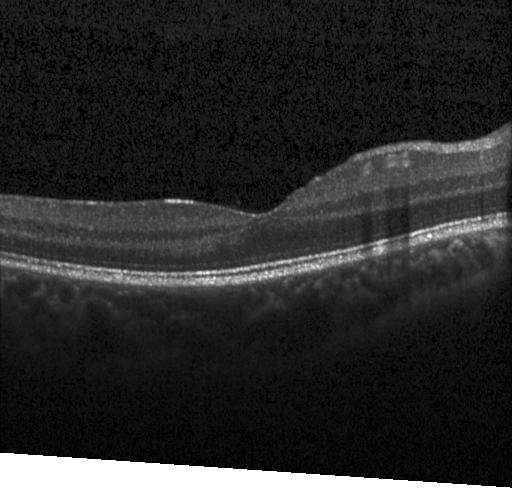

Spectral-domain OCT B-scan: no CNV, DME, or drusen.